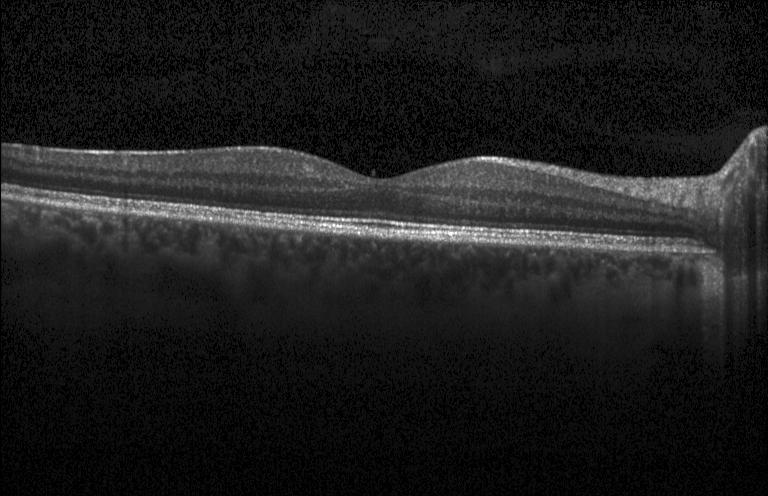

Macular scan · instrument: Heidelberg Spectralis · retinal OCT B-scan · spectral-domain OCT — Dx: no CNV, DME, or drusen.